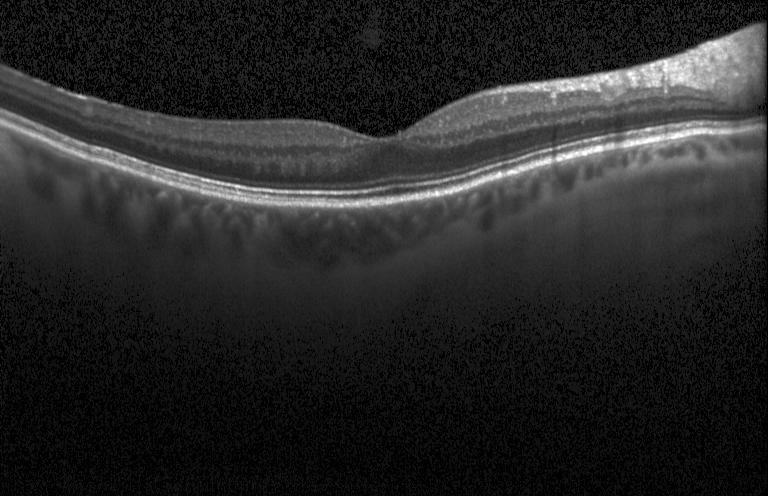

Through the macula; optical coherence tomography scan; Heidelberg Spectralis. Impression: no choroidal neovascularization, no diabetic macular edema, and no drusen.